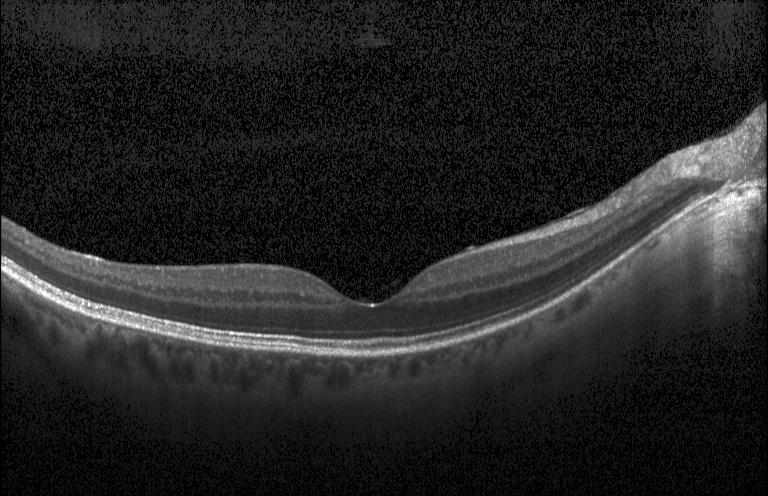

The scan shows no evidence of CNV, DME, or drusen.